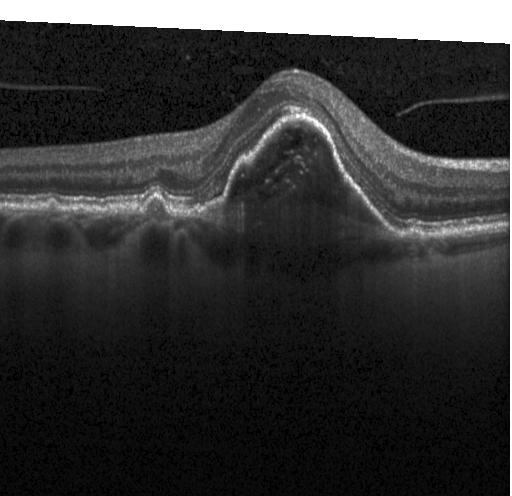

Spectral-domain OCT. Optical coherence tomography scan. Heidelberg Spectralis OCT system. Fovea-centered
Macular OCT: CNV.